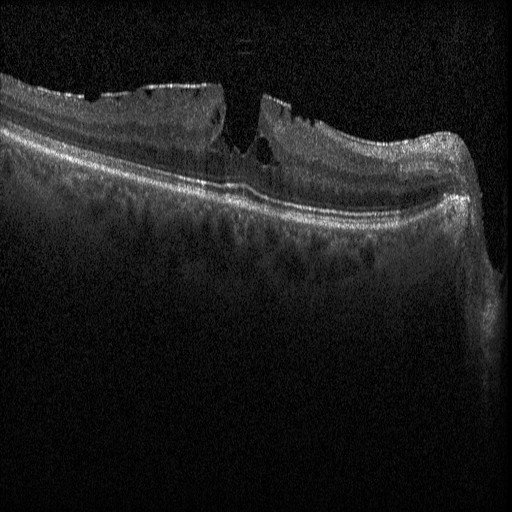

Macular OCT: diabetic macular edema.